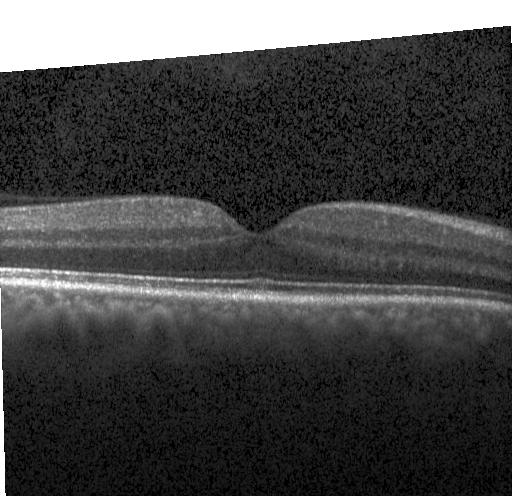 Finding: neither CNV, DME, nor drusen.